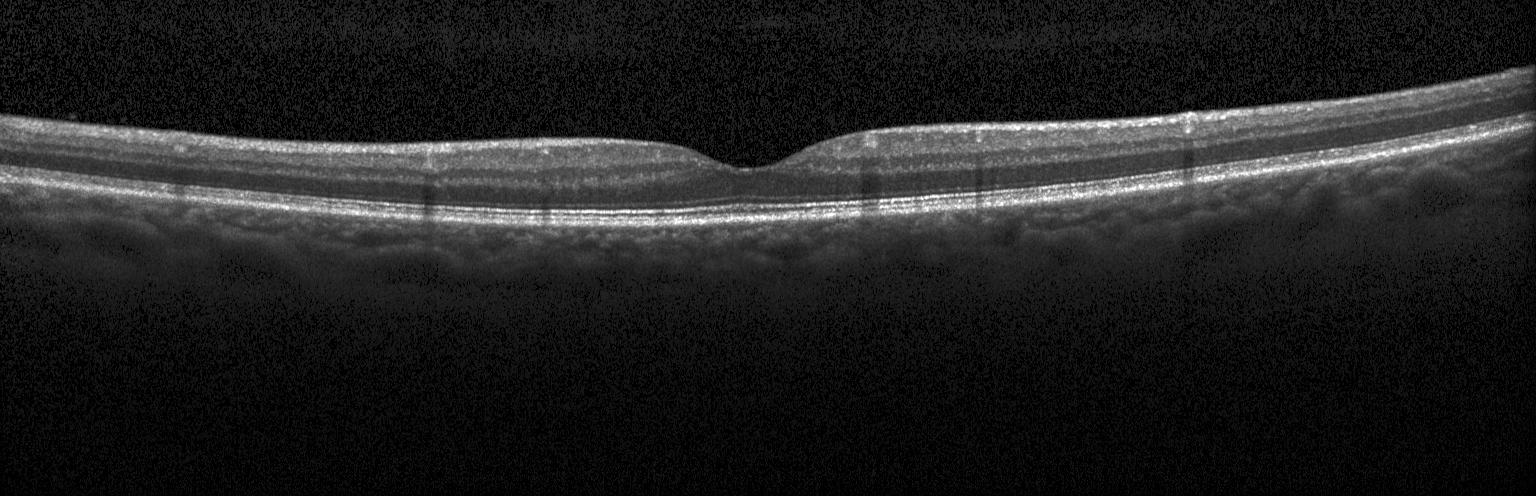
Impression: no evidence of CNV, DME, or drusen.